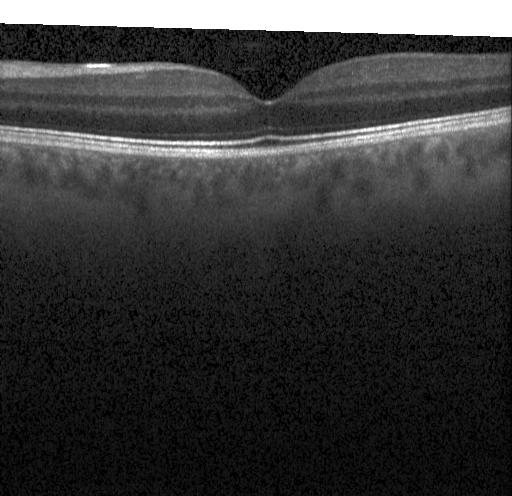

Fovea-centered · retinal OCT cross-section · acquired on a Heidelberg Spectralis · spectral-domain optical coherence tomography.
Finding: no evidence of choroidal neovascularization, diabetic macular edema, or drusen.